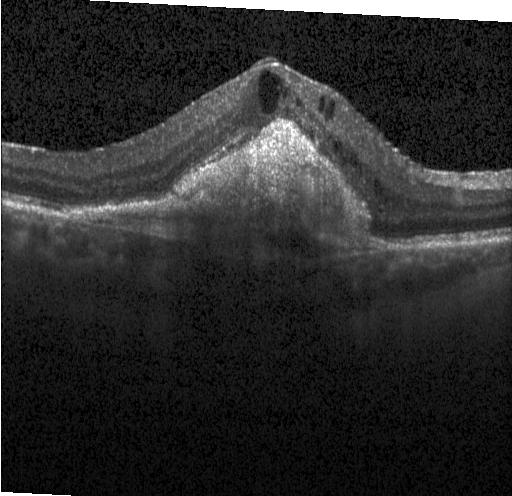 Fovea-centered · Heidelberg Spectralis · retinal OCT B-scan · SD-OCT.
Diagnosis: CNV.